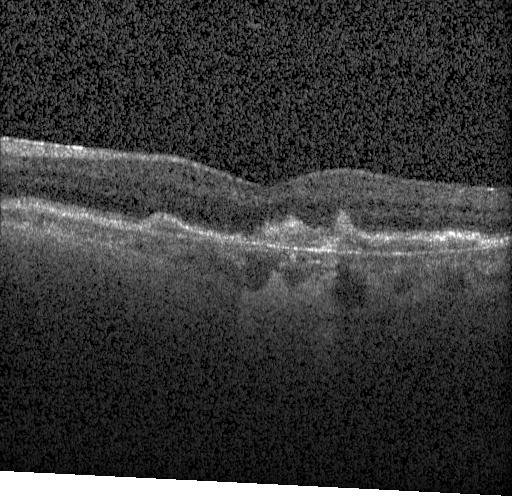
OCT B-scan — Assessment: a choroidal neovascular membrane.